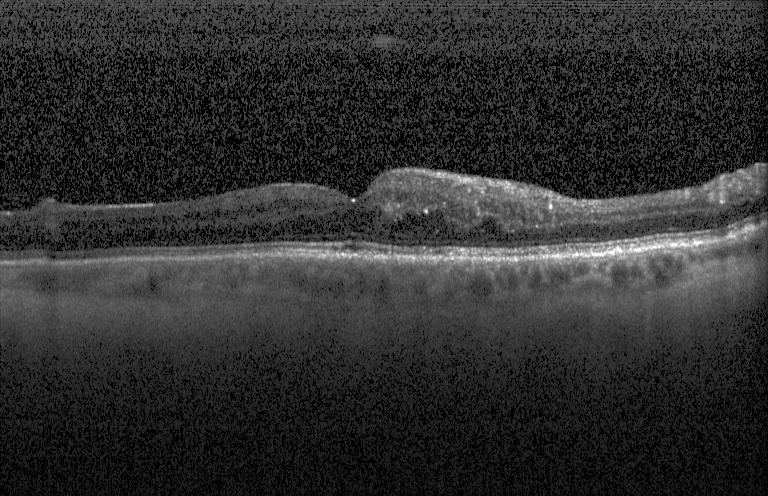
OCT finding: diabetic macular edema (DME).